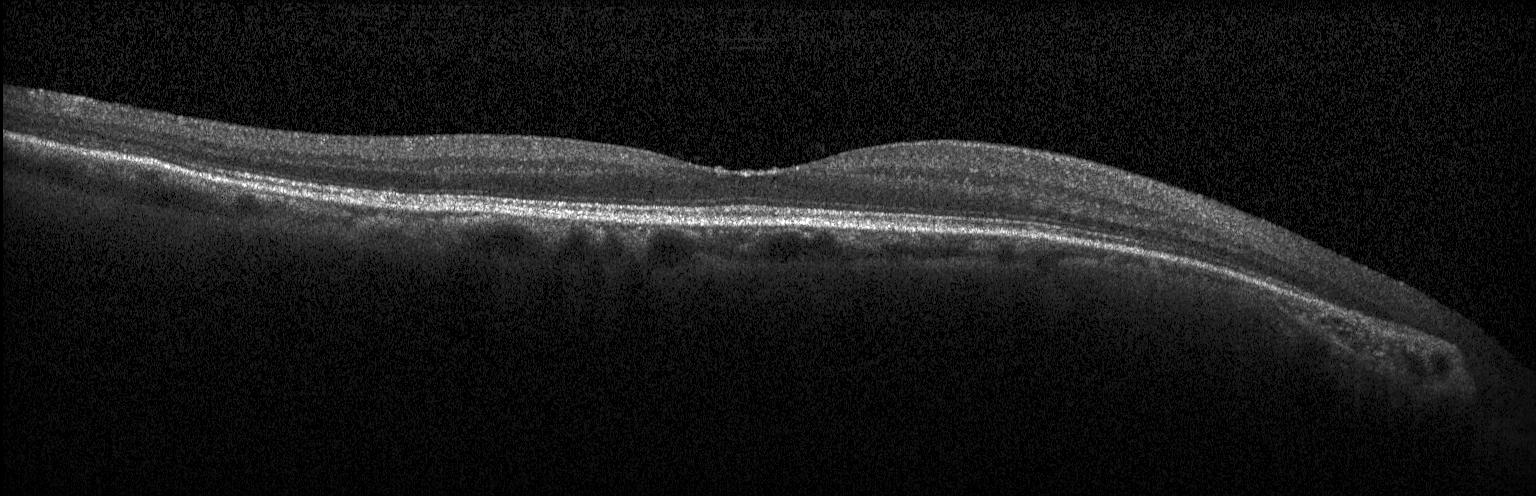 Centered on the fovea, Heidelberg Spectralis OCT system, OCT line scan.
Impression: no CNV, DME, or drusen.